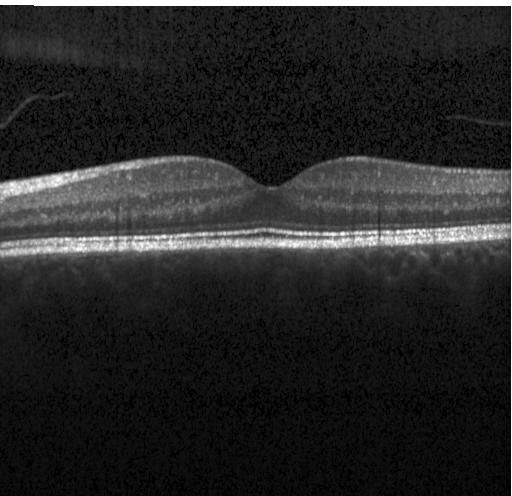
Instrument: Heidelberg Spectralis; optical coherence tomography scan; SD-OCT — Impression: no choroidal neovascularization, no diabetic macular edema, and no drusen.